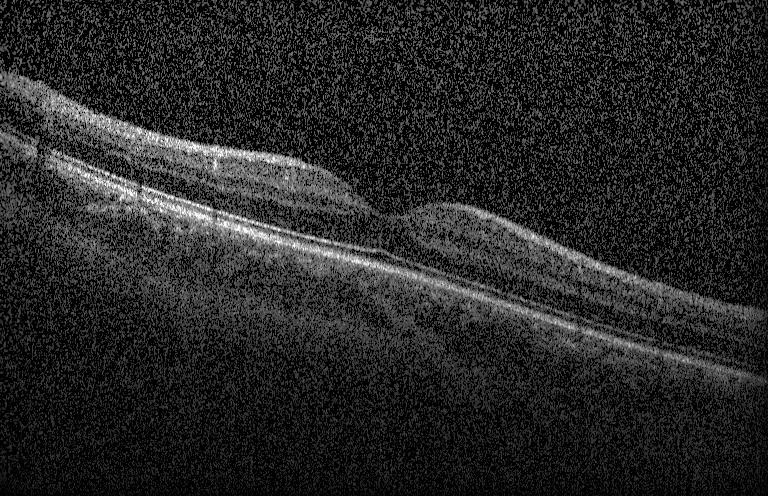
Spectral-domain optical coherence tomography; Heidelberg Spectralis; retinal OCT cross-section; macular scan.
Diagnosis: no CNV, no DME, and no drusen.